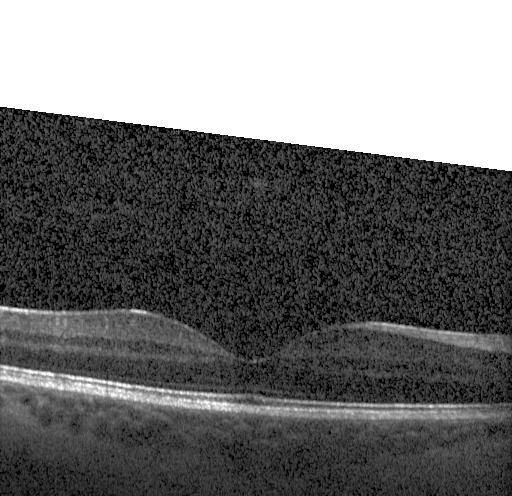
OCT B-scan · instrument: Heidelberg Spectralis
Finding: no evidence of CNV, DME, or drusen.